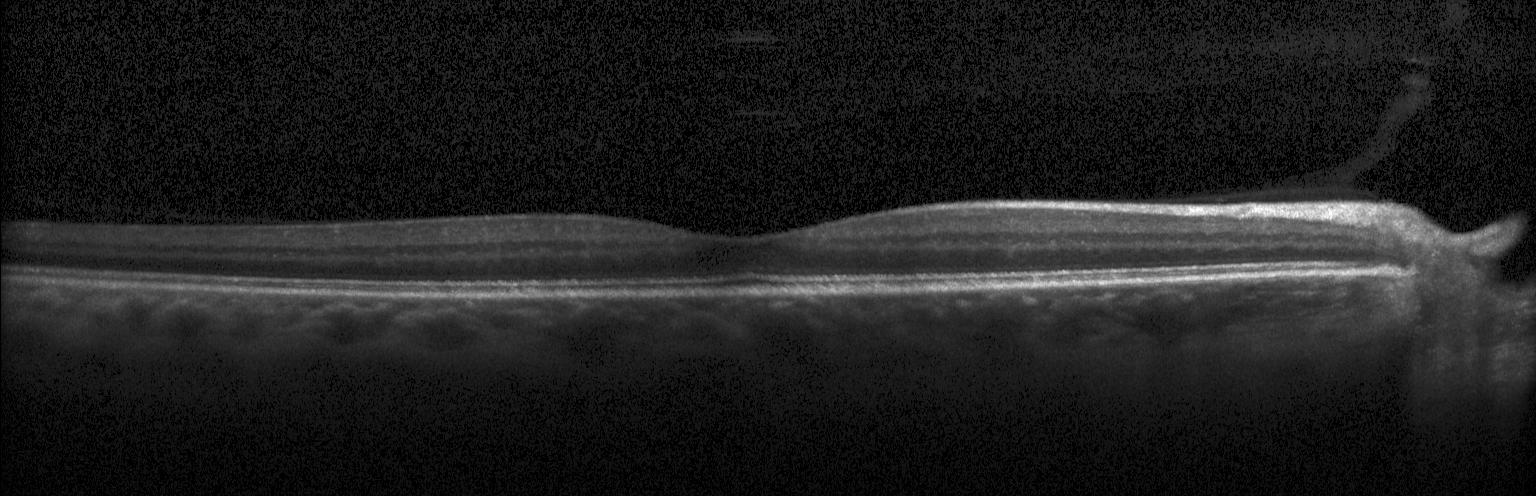
Spectral-domain OCT; centered on the fovea; retinal OCT cross-section
Finding: no evidence of CNV, DME, or drusen.